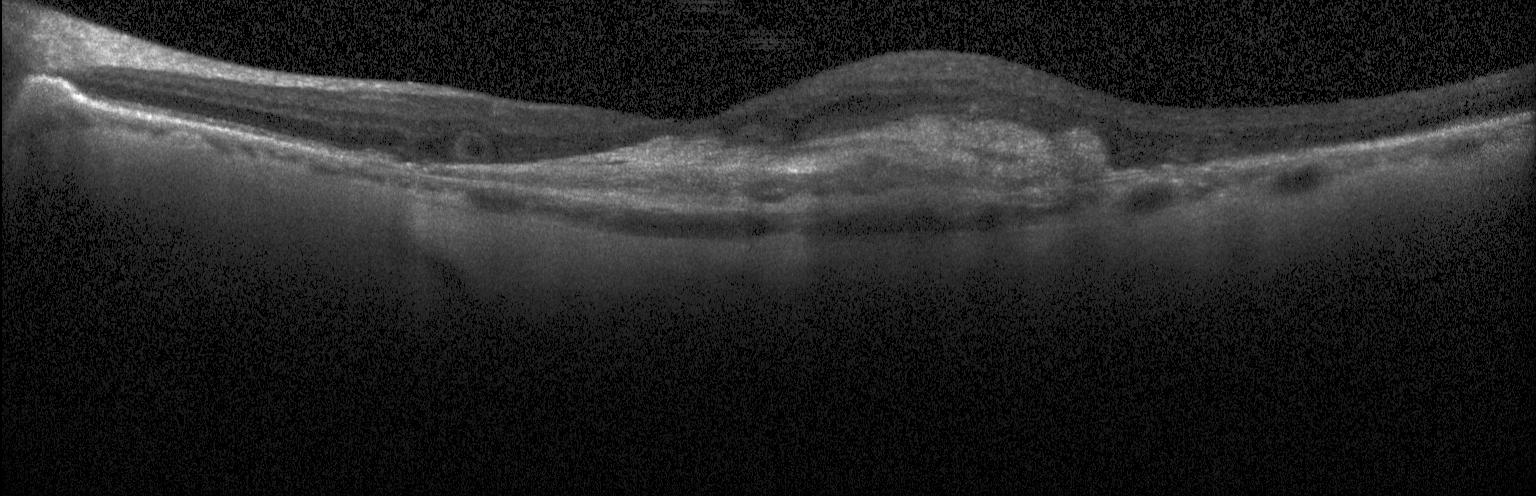

Dx: a choroidal neovascular membrane.